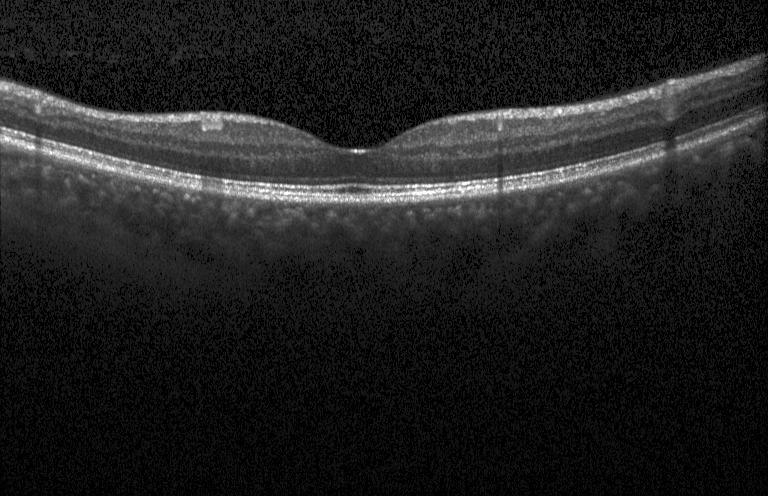

Diagnosis: neither CNV, DME, nor drusen.